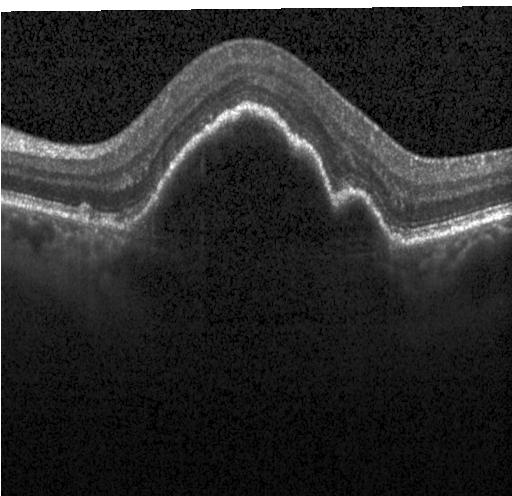
Optical coherence tomography B-scan
Impression: a choroidal neovascular membrane.